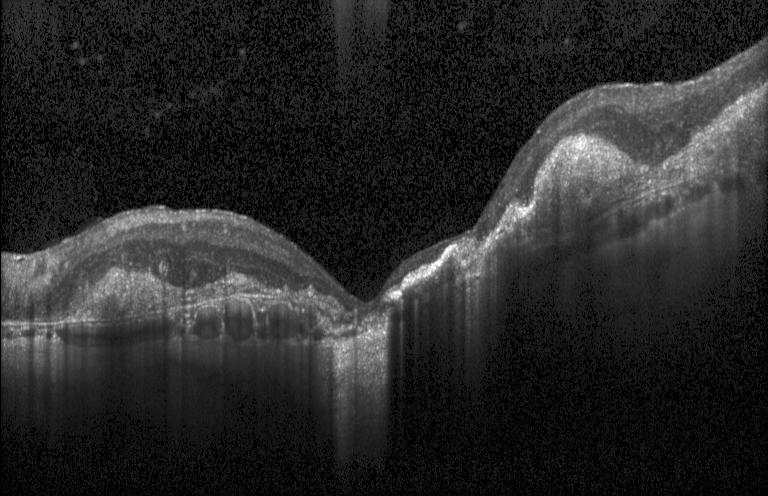
Optical coherence tomography B-scan. Impression: a choroidal neovascular membrane.